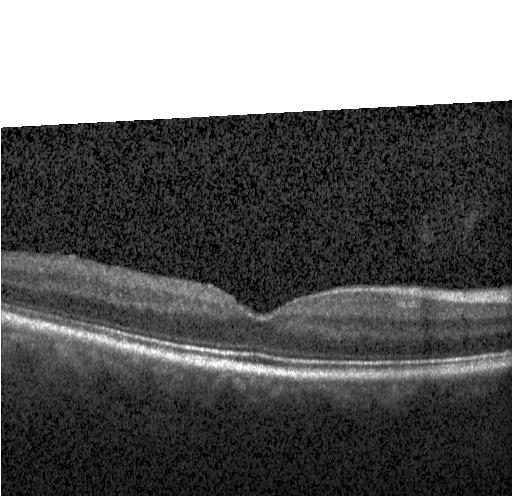
Dx: no CNV, DME, or drusen.